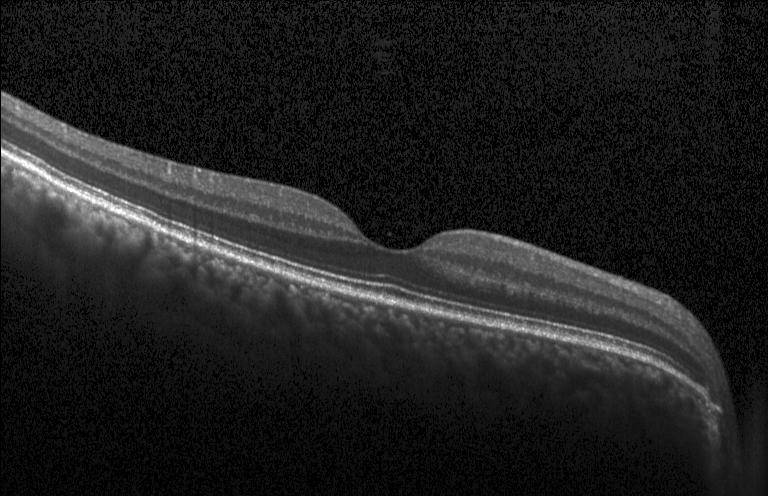 Dx: neither CNV, DME, nor drusen.